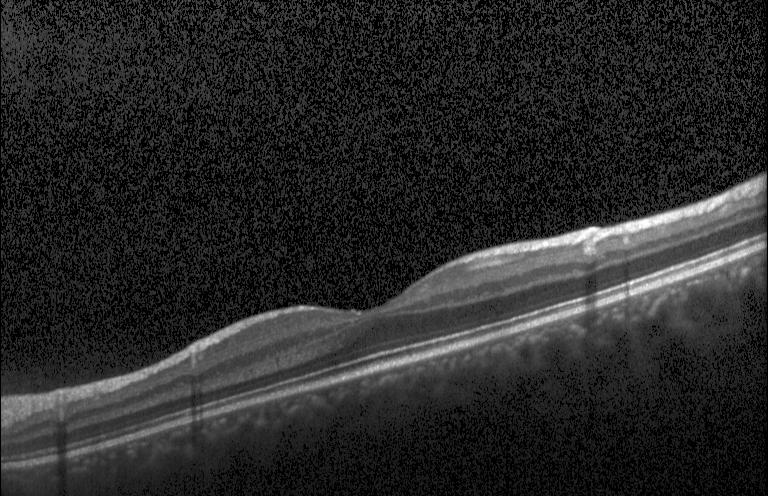 Impression: no choroidal neovascularization, no diabetic macular edema, and no drusen.